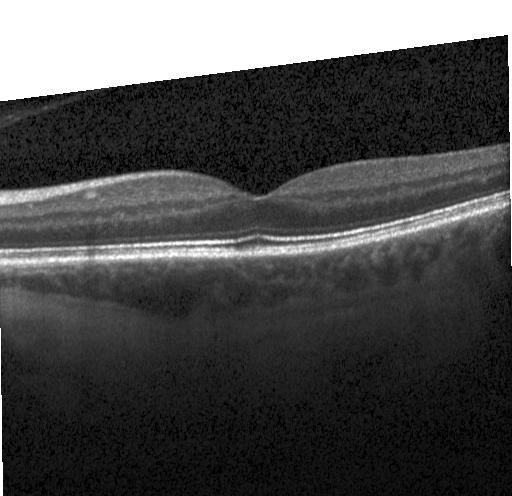
Impression: no evidence of CNV, DME, or drusen.